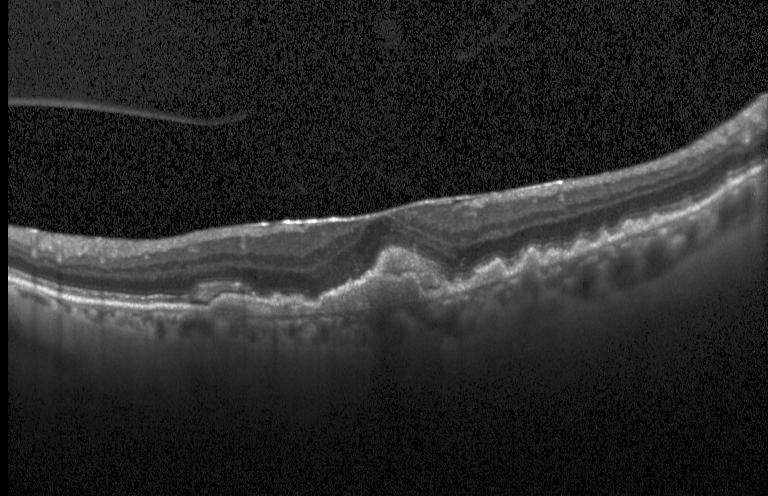

Retinal OCT B-scan
Finding: a choroidal neovascular membrane.